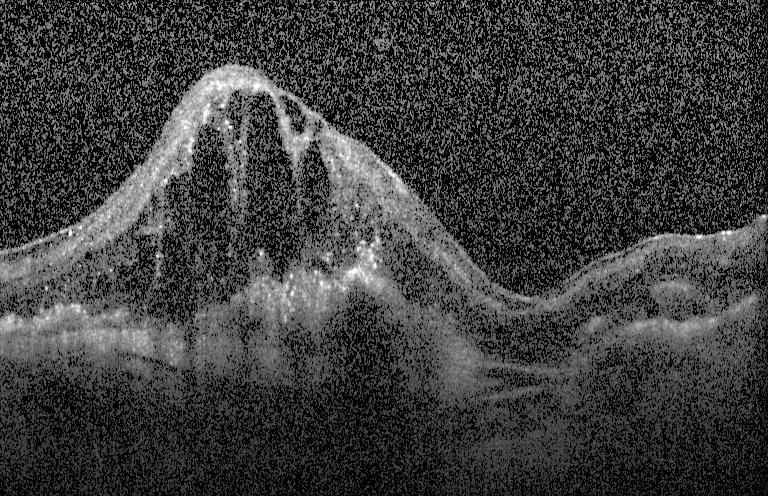
Instrument: Heidelberg Spectralis · horizontal scan through the fovea · retinal OCT cross-section
Finding: a choroidal neovascular membrane.